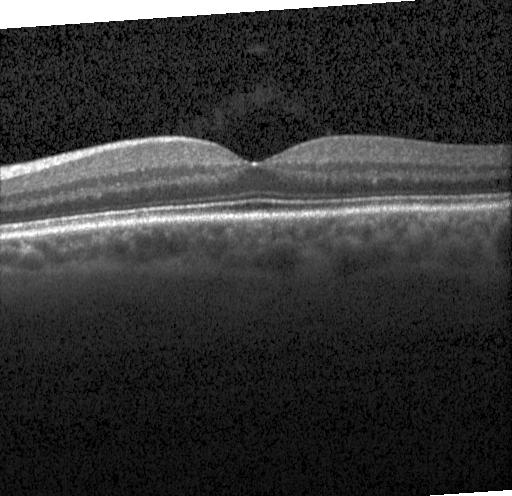
Through the macula · OCT line scan — OCT finding: neither CNV, DME, nor drusen.